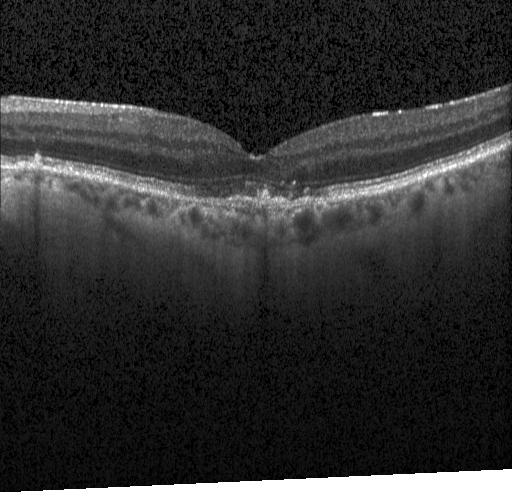 Spectral-domain OCT B-scan: choroidal neovascularization (CNV).